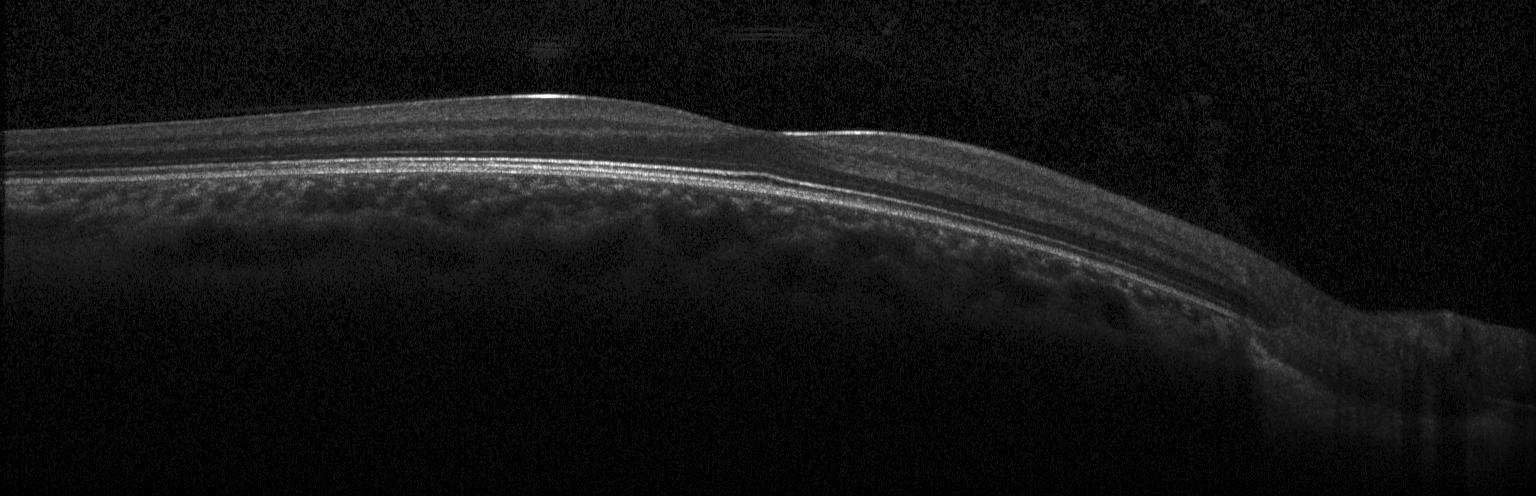
The scan shows neither choroidal neovascularization, diabetic macular edema, nor drusen.